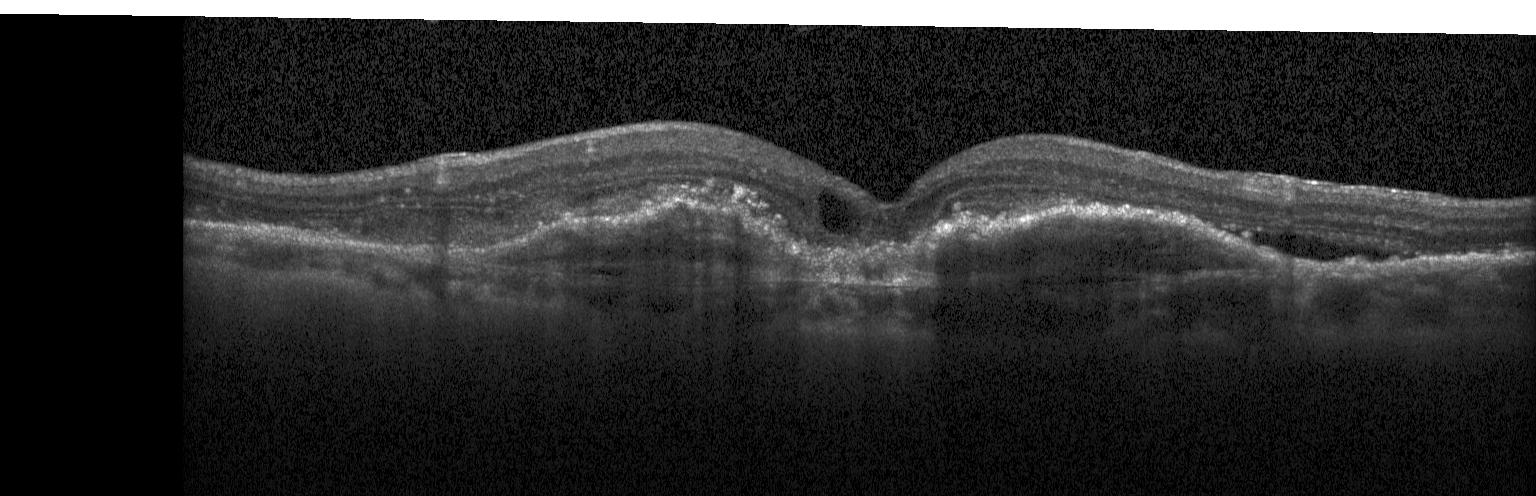
Optical coherence tomography B-scan. Spectral-domain OCT.
Diagnosis: a choroidal neovascular membrane.